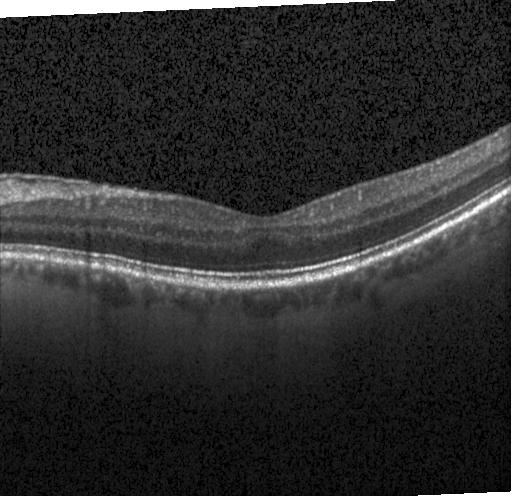 Diagnosis: no choroidal neovascularization, no diabetic macular edema, and no drusen.